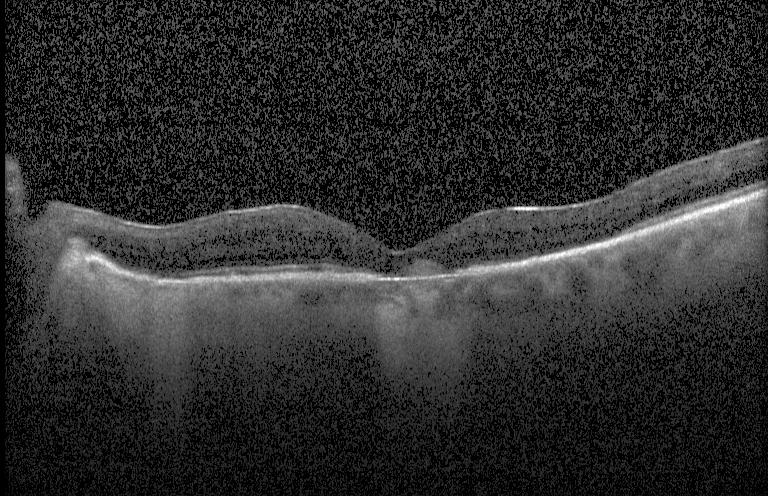 Finding: a choroidal neovascular membrane.